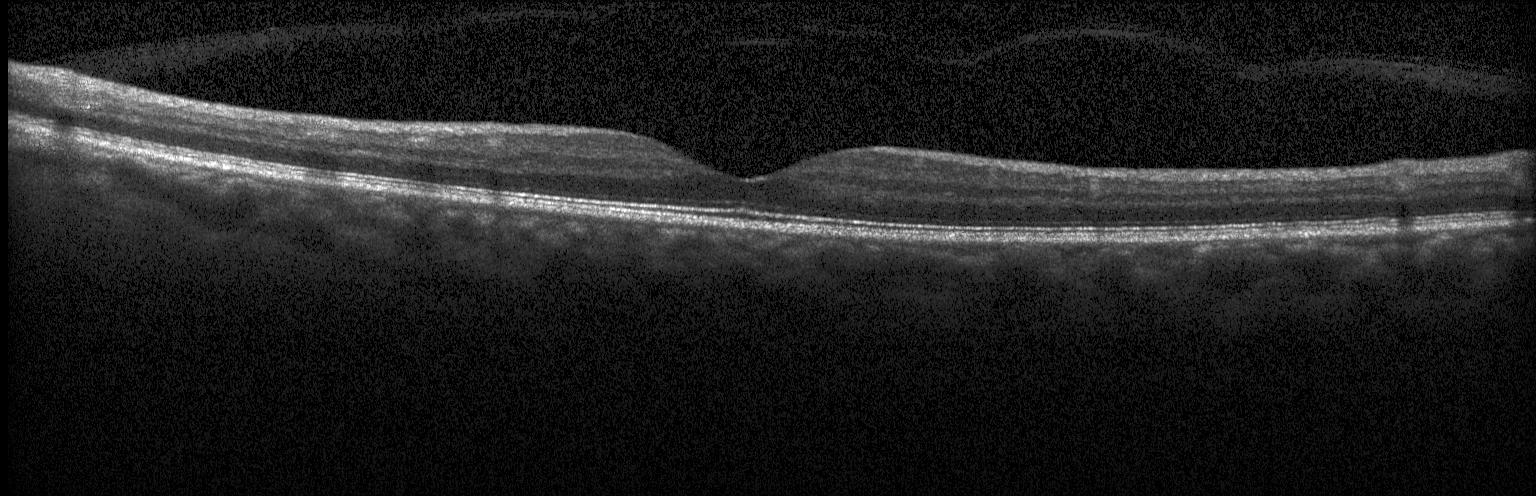
Spectral-domain OCT B-scan: no CNV, no DME, and no drusen.